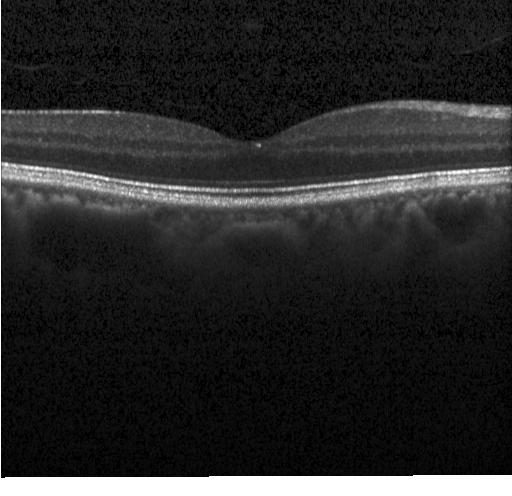 Retinal OCT cross-section showing no evidence of choroidal neovascularization, diabetic macular edema, or drusen.